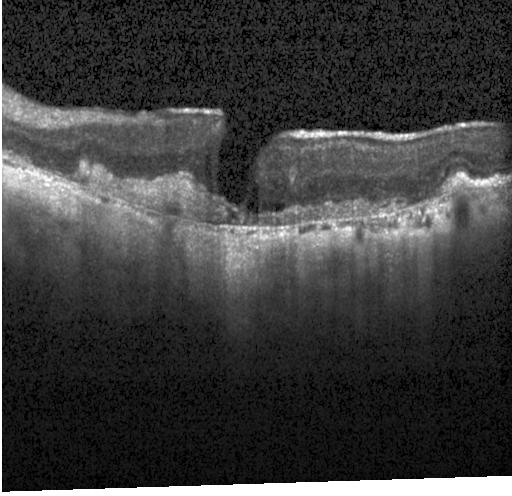

Diagnosis: choroidal neovascularization (CNV).